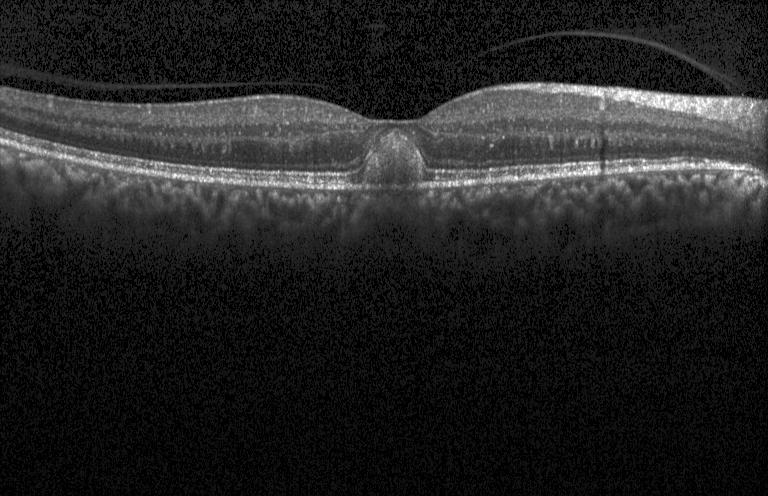 Retinal OCT cross-section; Heidelberg Spectralis OCT system — Diagnosis: a choroidal neovascular membrane.